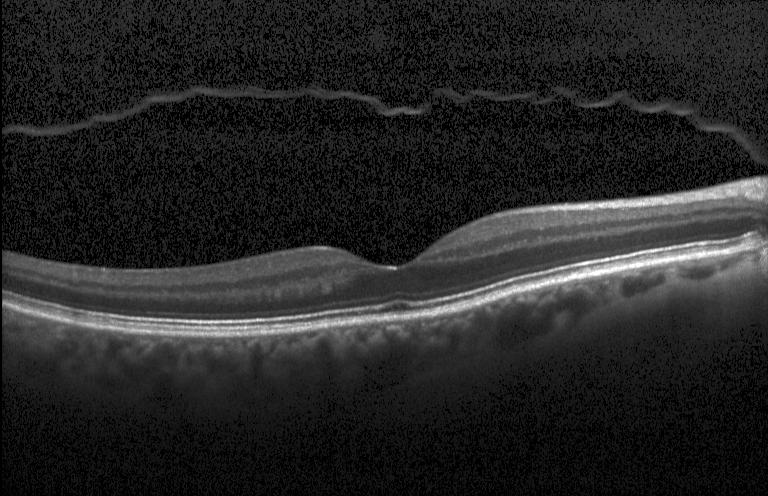

Macular OCT: no choroidal neovascularization, no diabetic macular edema, and no drusen.